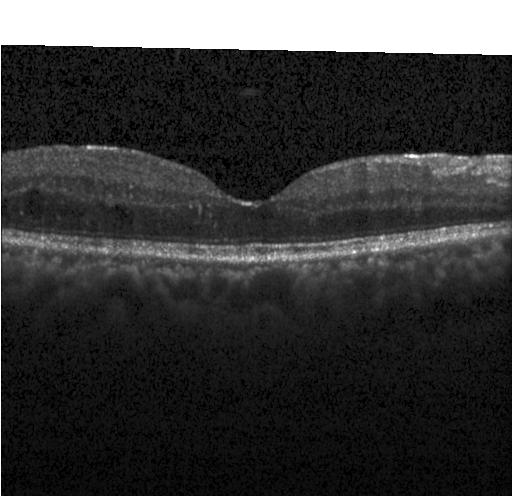

Impression: diabetic macular edema.